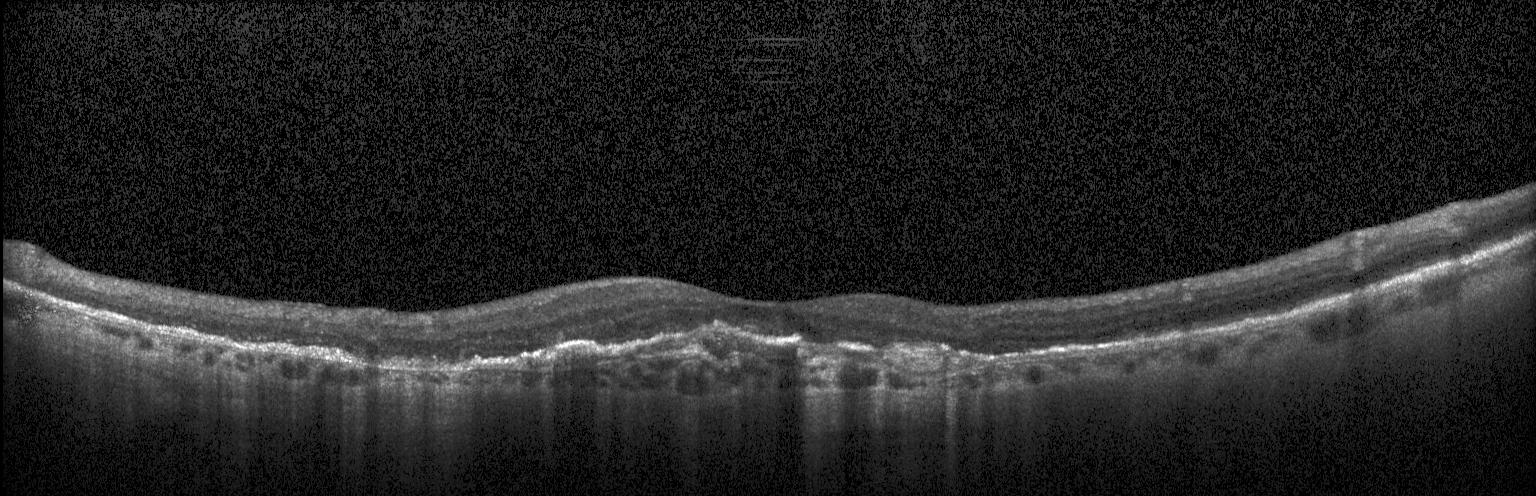

OCT finding: a choroidal neovascular membrane.